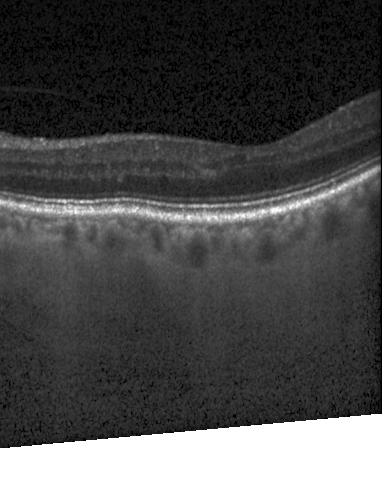

Diagnosis: no CNV, no DME, and no drusen.